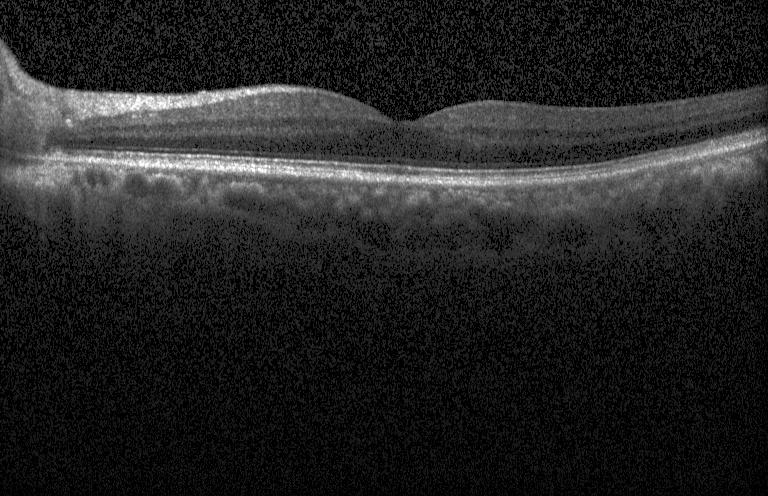

Retinal OCT B-scan — Finding: no CNV, DME, or drusen.